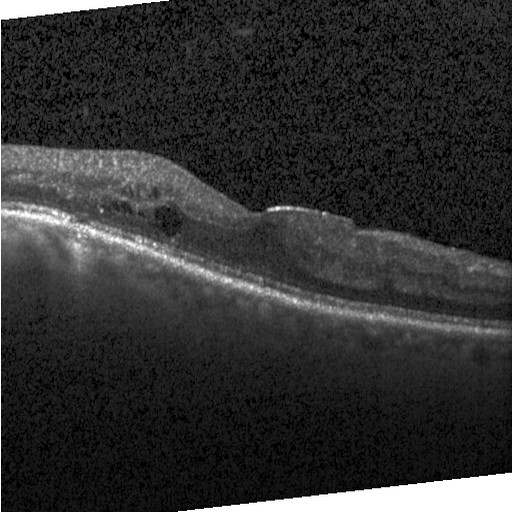 Spectral-domain OCT; retinal OCT cross-section. Dx: diabetic macular edema (DME).